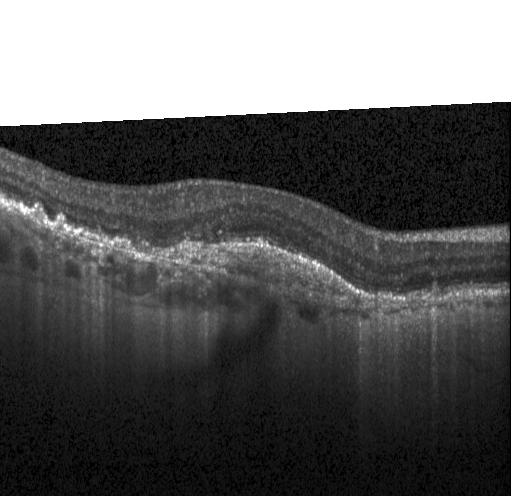

Through the macula. Heidelberg Spectralis. Optical coherence tomography scan.
Finding: a choroidal neovascular membrane.